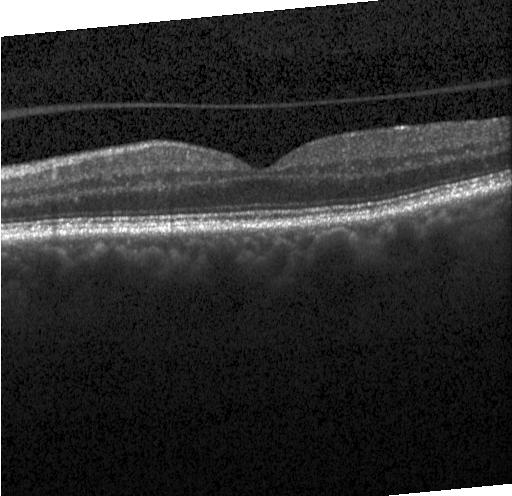 Fovea-centered. Optical coherence tomography scan. Spectral-domain OCT.
Macular OCT: neither CNV, DME, nor drusen.